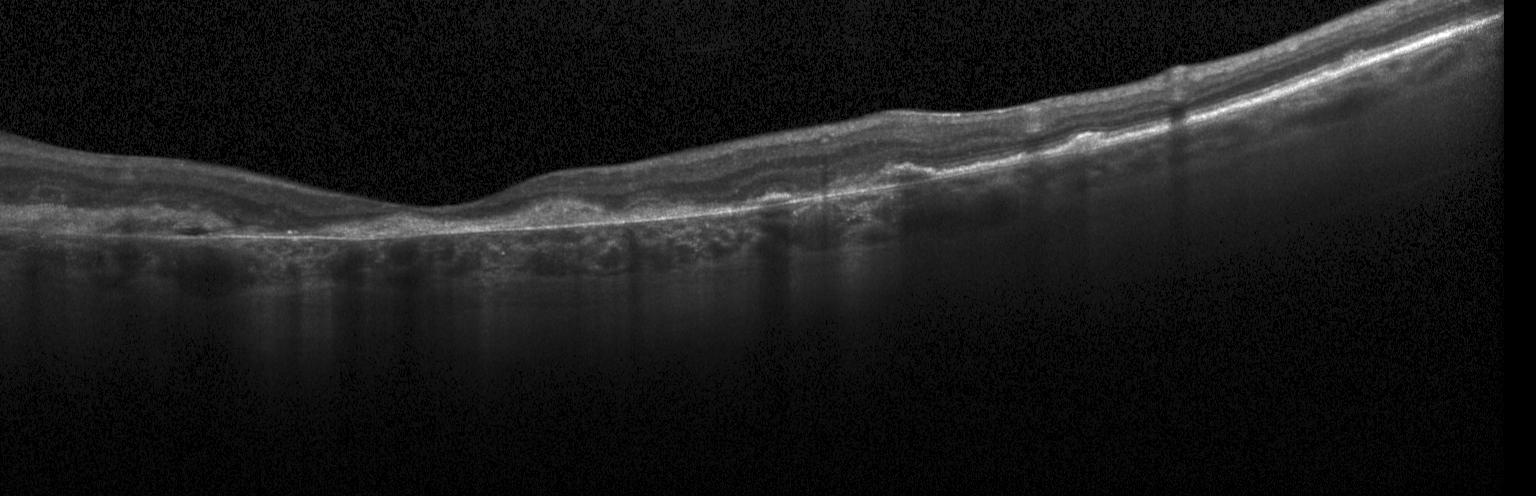 Retinal OCT cross-section
Impression: a choroidal neovascular membrane.